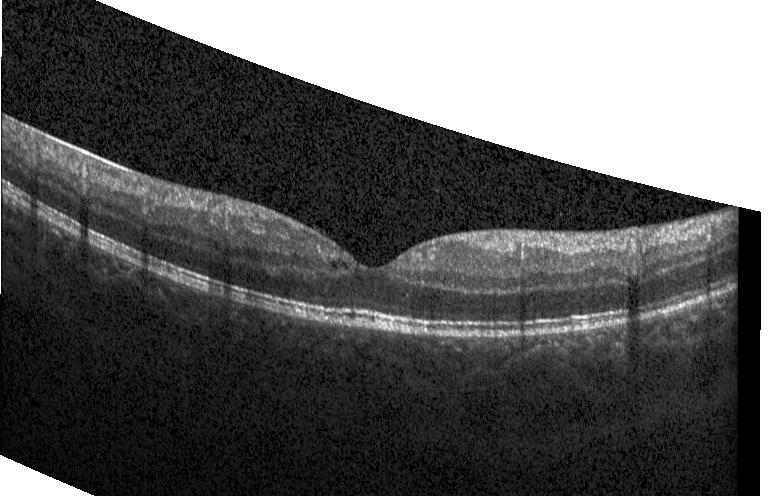

Diagnosis: diabetic macular edema (DME).